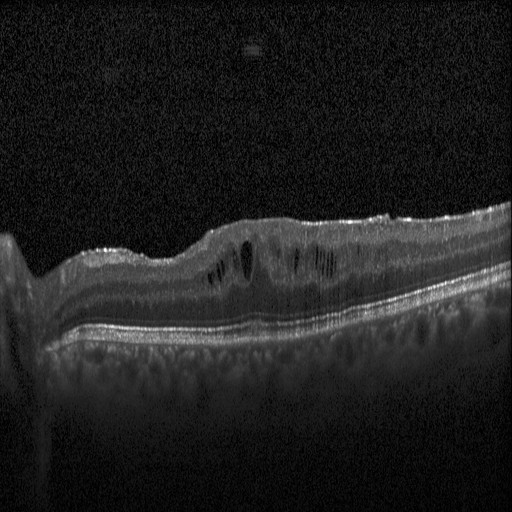 DME.